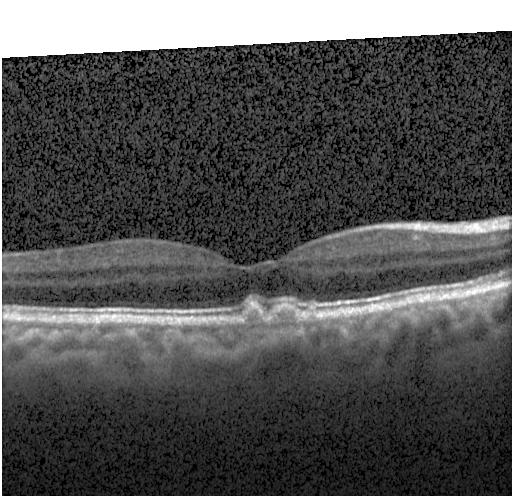 Diagnosis: drusen.